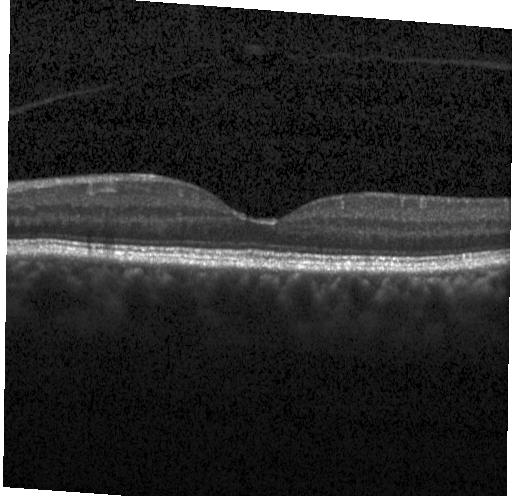
OCT line scan — This B-scan demonstrates no CNV, no DME, and no drusen.